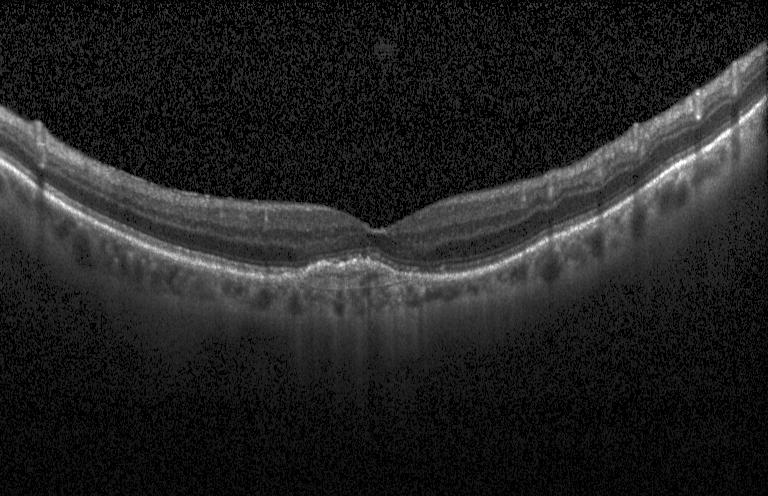 A choroidal neovascular membrane.